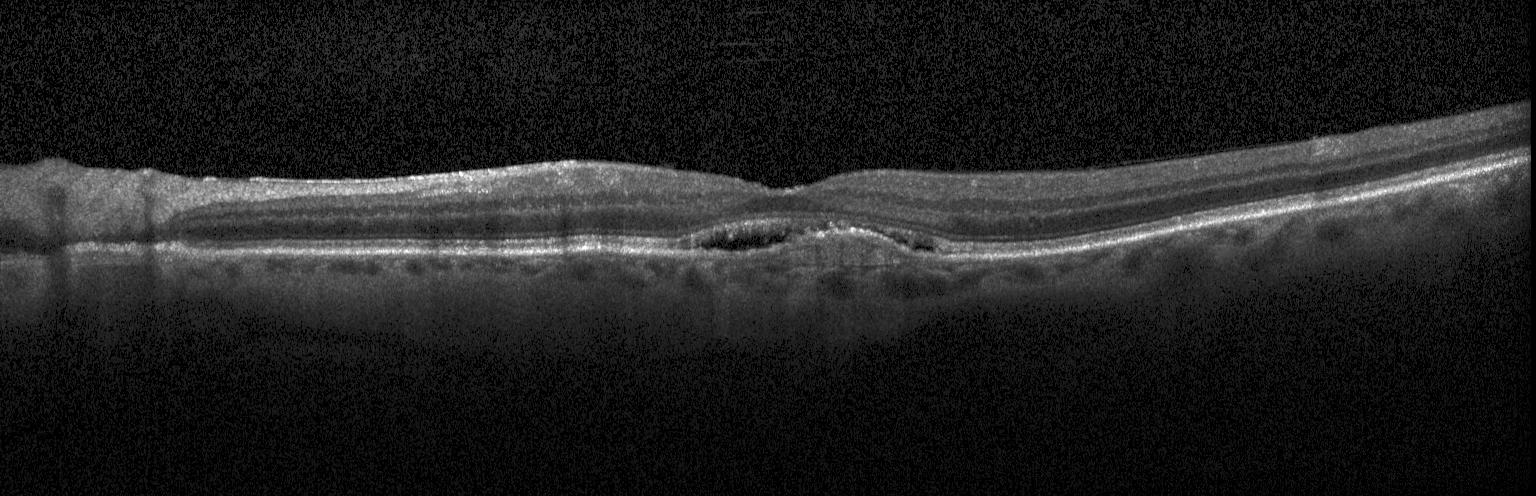 Retinal OCT cross-section showing choroidal neovascularization (CNV).